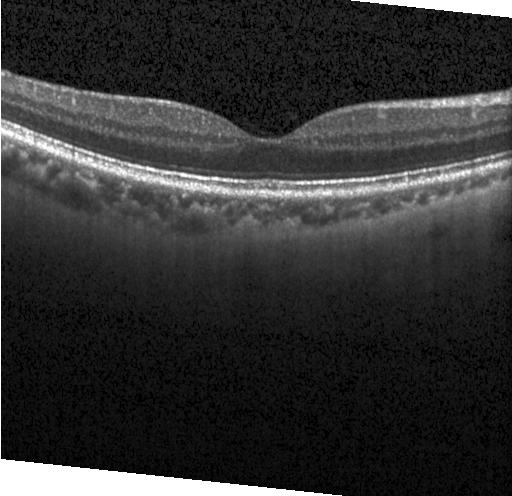

Neither choroidal neovascularization, diabetic macular edema, nor drusen.